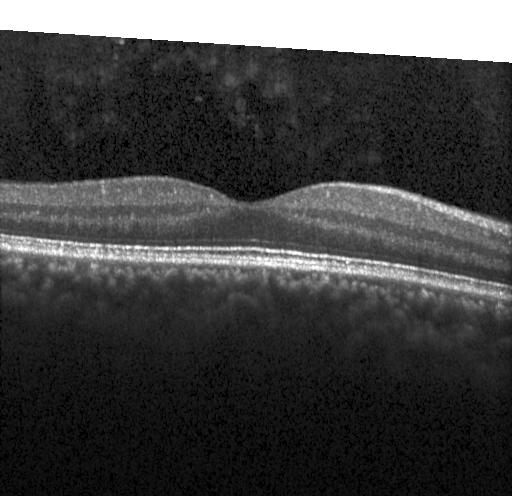
Through the macula; spectral-domain OCT; Heidelberg Spectralis OCT system; OCT B-scan
Macular OCT: no choroidal neovascularization, no diabetic macular edema, and no drusen.